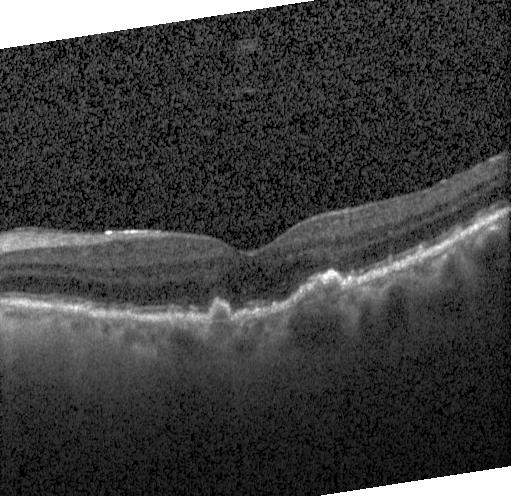
Macular OCT: a choroidal neovascular membrane.